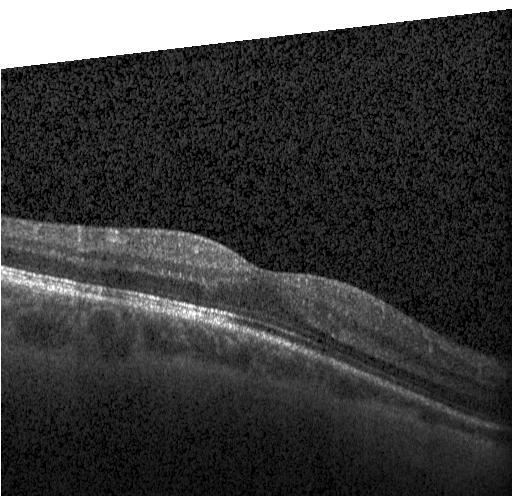 OCT finding: no choroidal neovascularization, no diabetic macular edema, and no drusen.